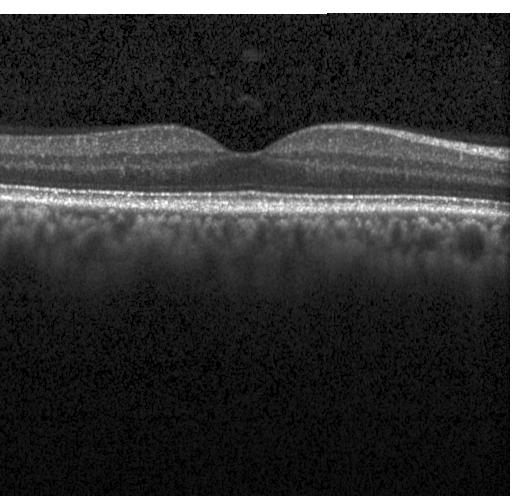

Optical coherence tomography scan · horizontal scan through the fovea · SD-OCT · Heidelberg Spectralis — Assessment: neither choroidal neovascularization, diabetic macular edema, nor drusen.